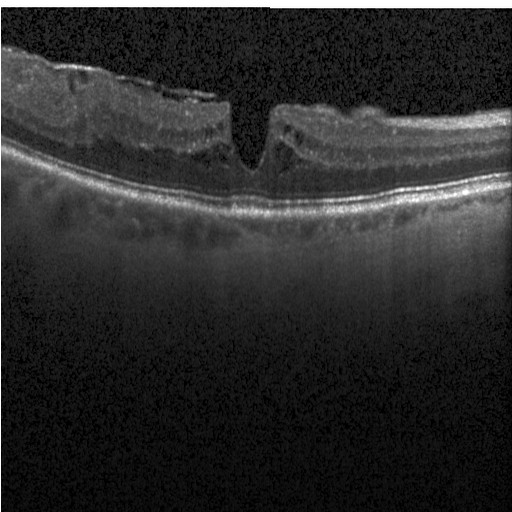
SD-OCT, acquired on a Heidelberg Spectralis, optical coherence tomography scan.
Impression: diabetic macular edema (DME).